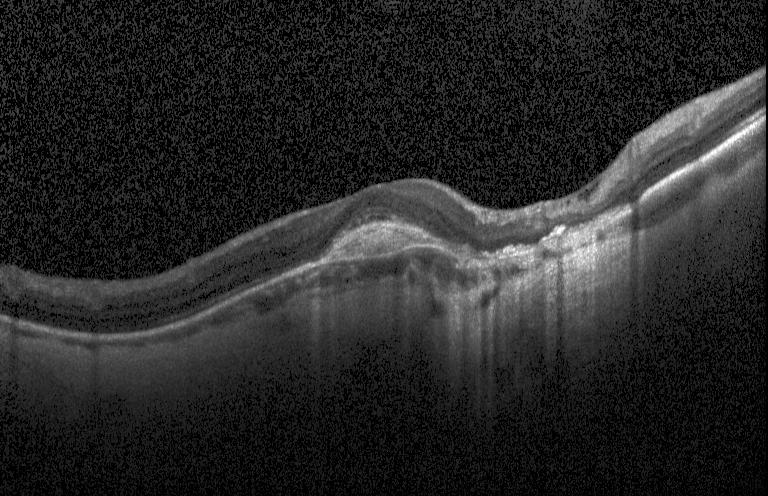 Spectral-domain OCT B-scan: choroidal neovascularization (CNV).